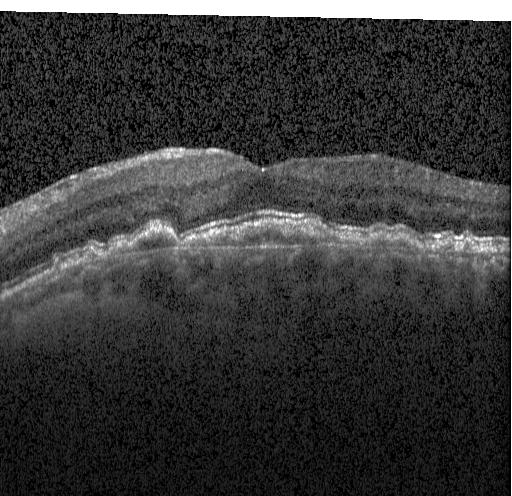 Optical coherence tomography B-scan. A choroidal neovascular membrane.